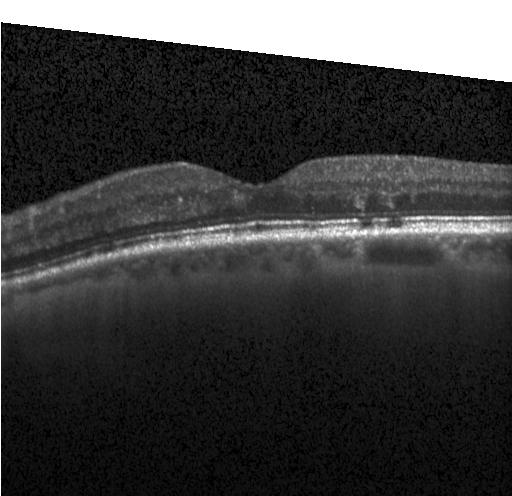 Spectral-domain OCT B-scan: diabetic macular edema.